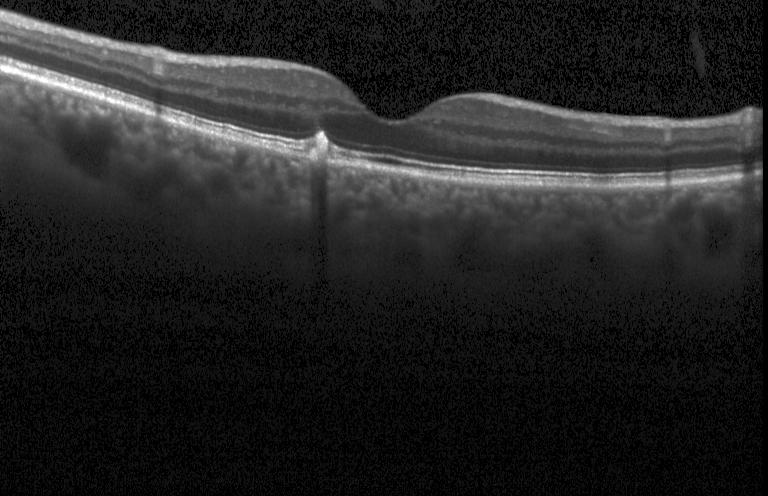
Diagnosis: drusen.